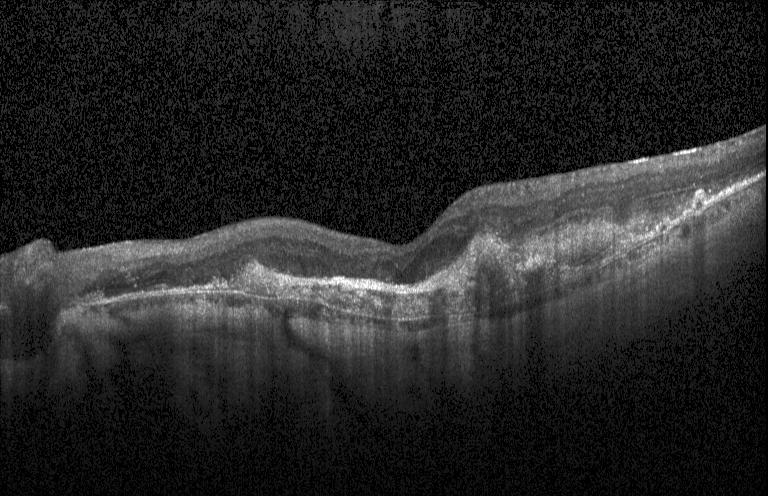 Finding: a choroidal neovascular membrane.